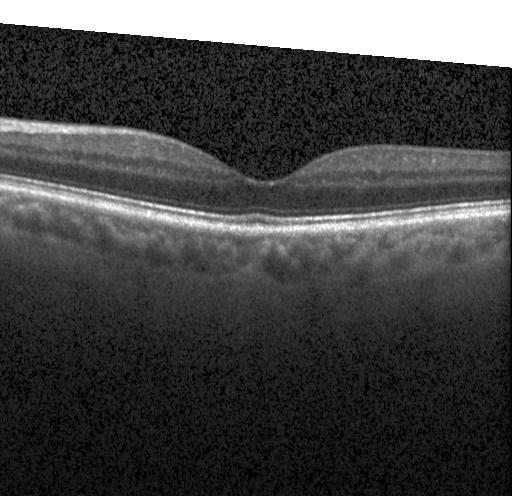 OCT line scan — No choroidal neovascularization, no diabetic macular edema, and no drusen.